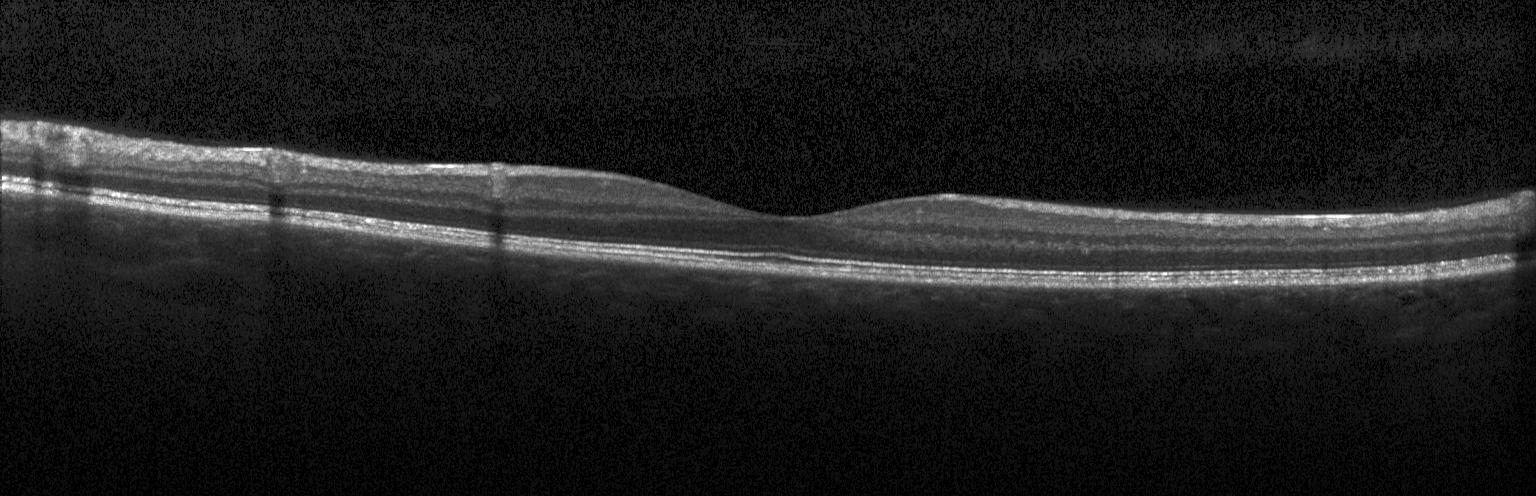 Impression: no choroidal neovascularization, no diabetic macular edema, and no drusen.